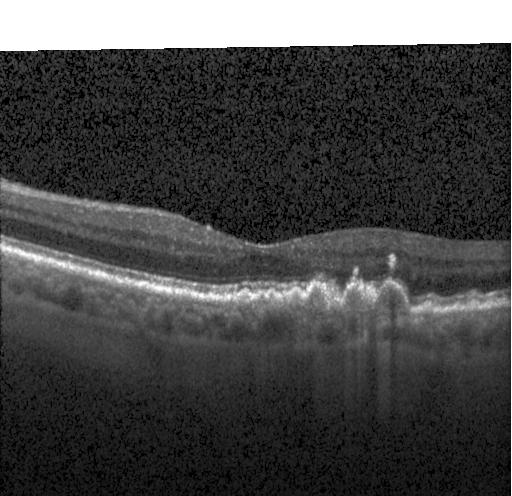

Retinal OCT B-scan; acquired on a Heidelberg Spectralis — Dx: drusen.